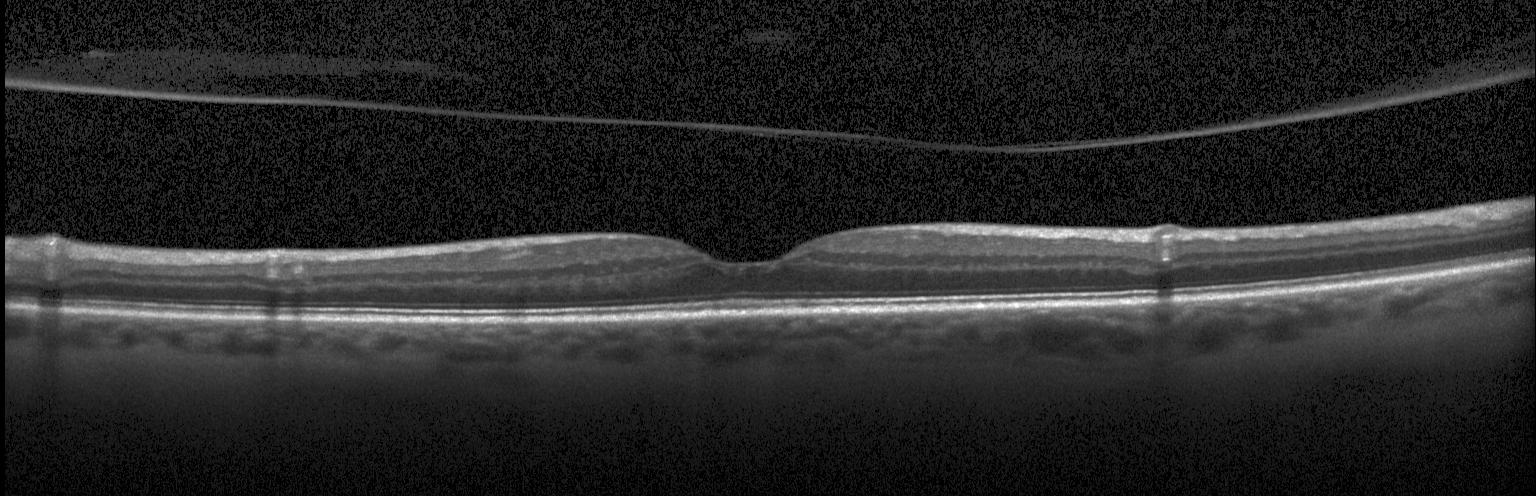
Assessment: neither CNV, DME, nor drusen.